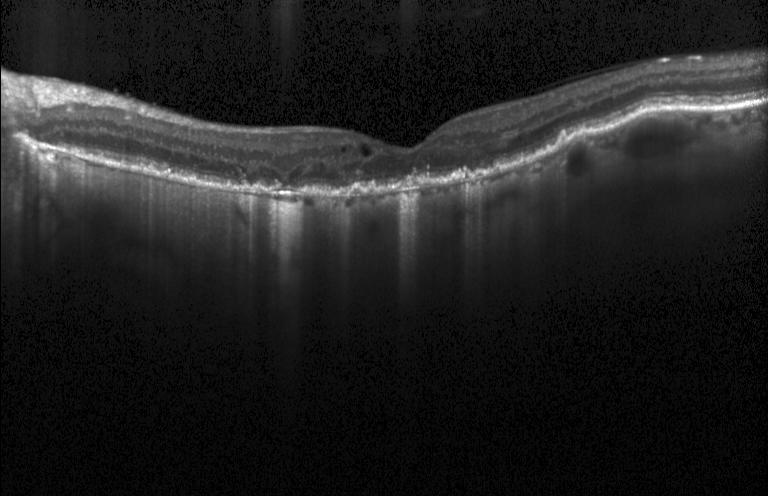
This B-scan demonstrates a choroidal neovascular membrane.